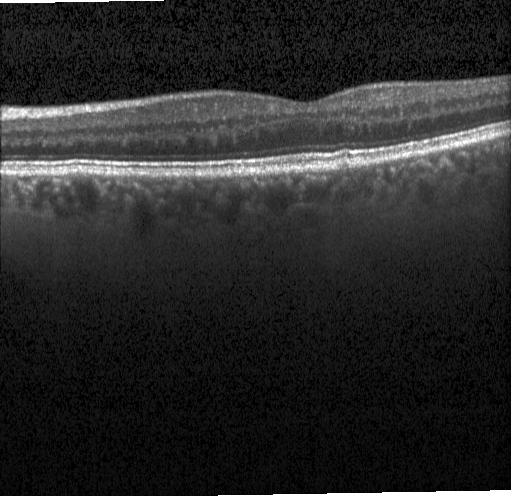 SD-OCT, optical coherence tomography B-scan, through the macula, Heidelberg Spectralis.
Impression: no CNV, no DME, and no drusen.